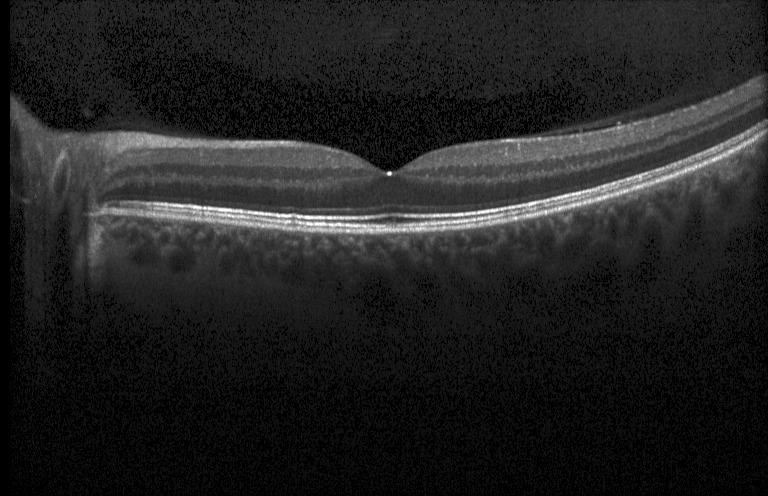

Heidelberg Spectralis OCT system; optical coherence tomography B-scan — Finding: neither choroidal neovascularization, diabetic macular edema, nor drusen.